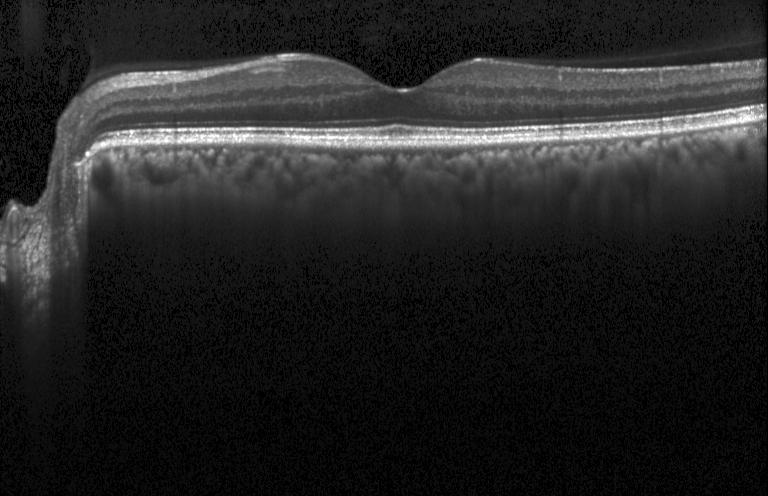

Finding: no choroidal neovascularization, no diabetic macular edema, and no drusen.